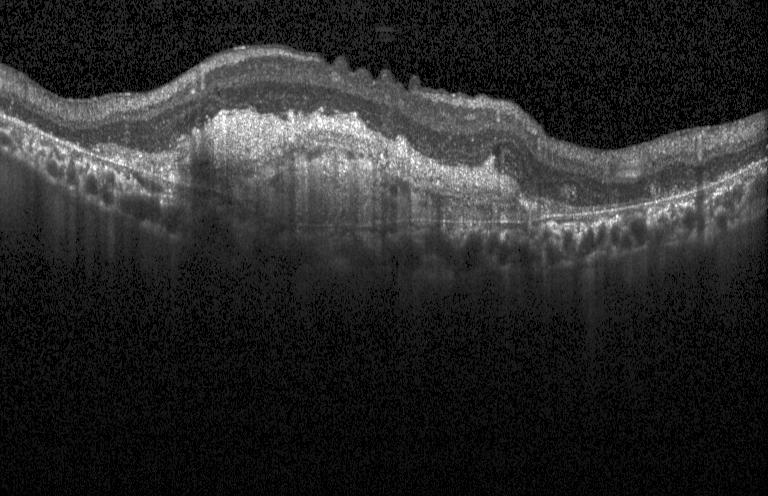
Diagnosis: choroidal neovascularization (CNV).